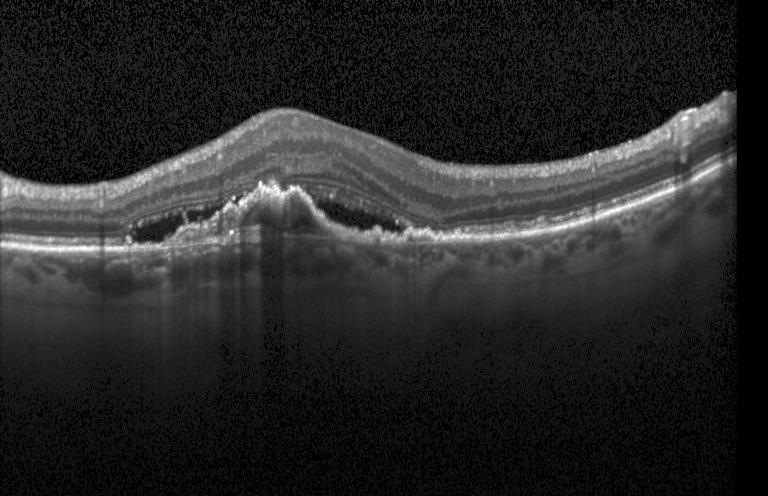 Retinal OCT cross-section, fovea-centered, Heidelberg Spectralis.
Assessment: choroidal neovascularization (CNV).